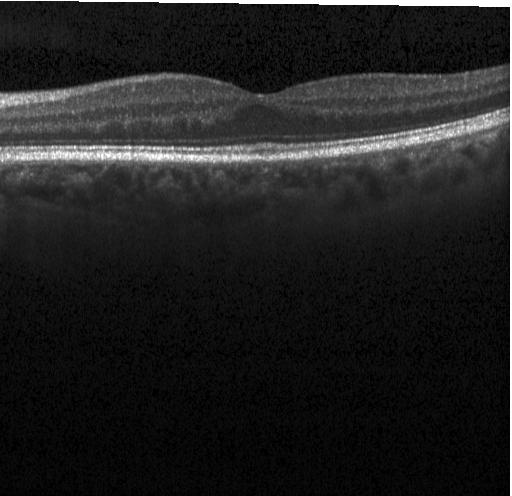
Heidelberg Spectralis OCT system · spectral-domain optical coherence tomography · macular scan · retinal OCT B-scan. Finding: no choroidal neovascularization, diabetic macular edema, or drusen.